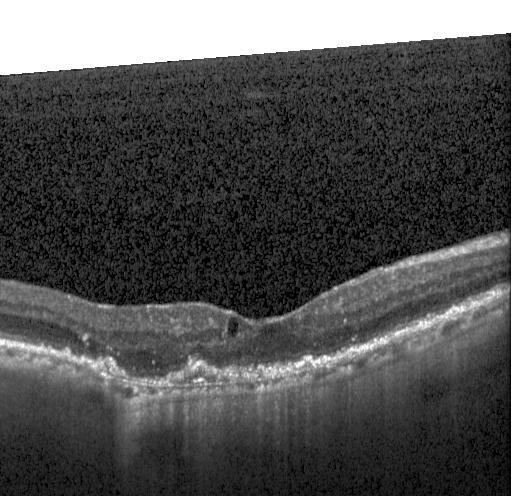

OCT B-scan · SD-OCT · through the macula.
Assessment: a choroidal neovascular membrane.